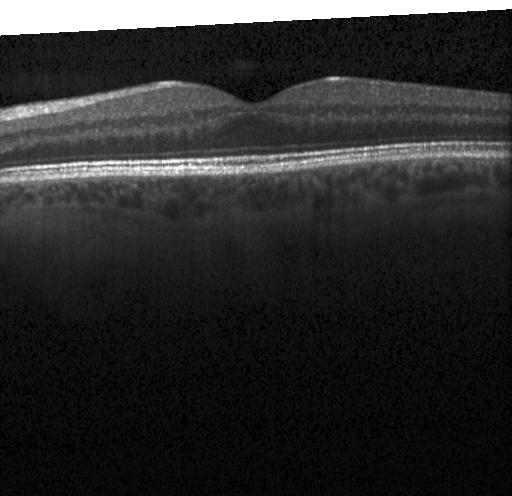 OCT line scan — Neither CNV, DME, nor drusen.